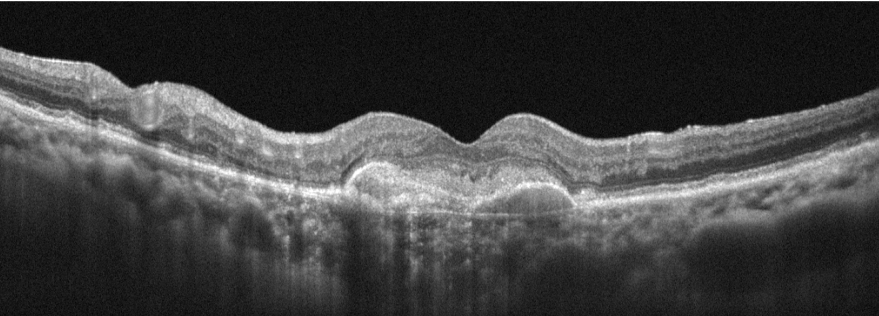 Optical coherence tomography scan. Impression: AMD.